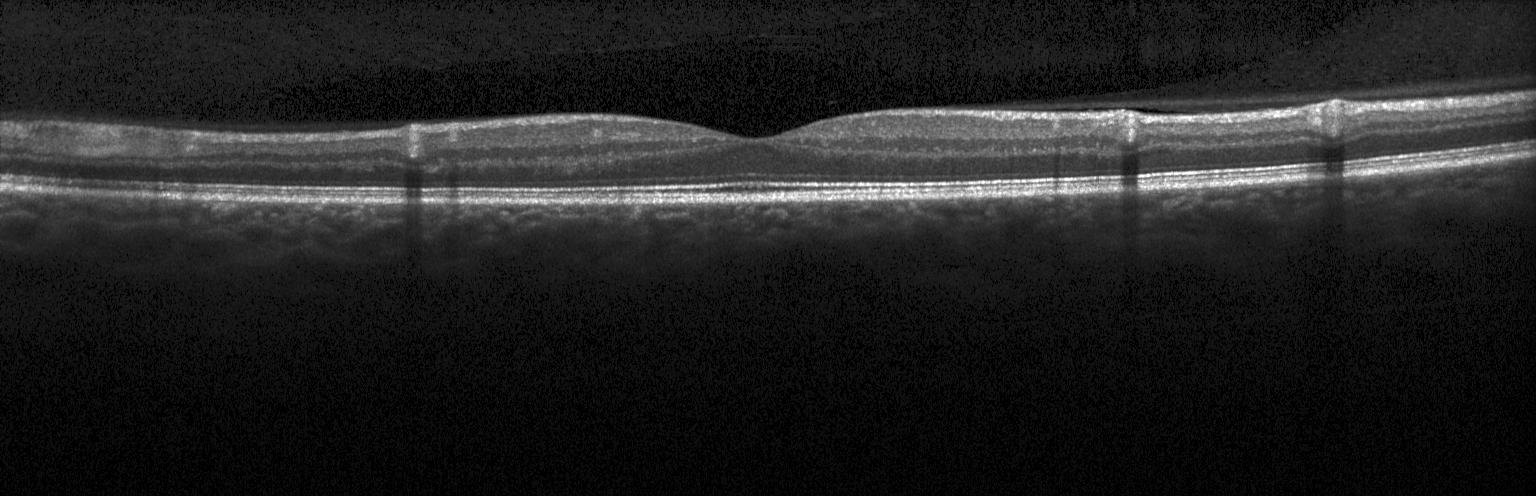 Impression: no evidence of choroidal neovascularization, diabetic macular edema, or drusen.